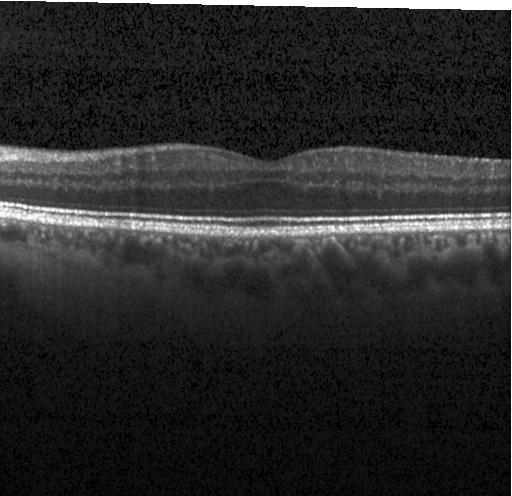 Spectral-domain optical coherence tomography · optical coherence tomography B-scan.
Diagnosis: no CNV, no DME, and no drusen.